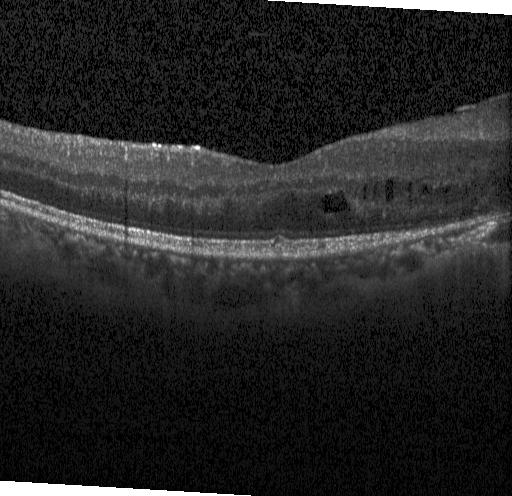 Retinal OCT cross-section showing diabetic macular edema.